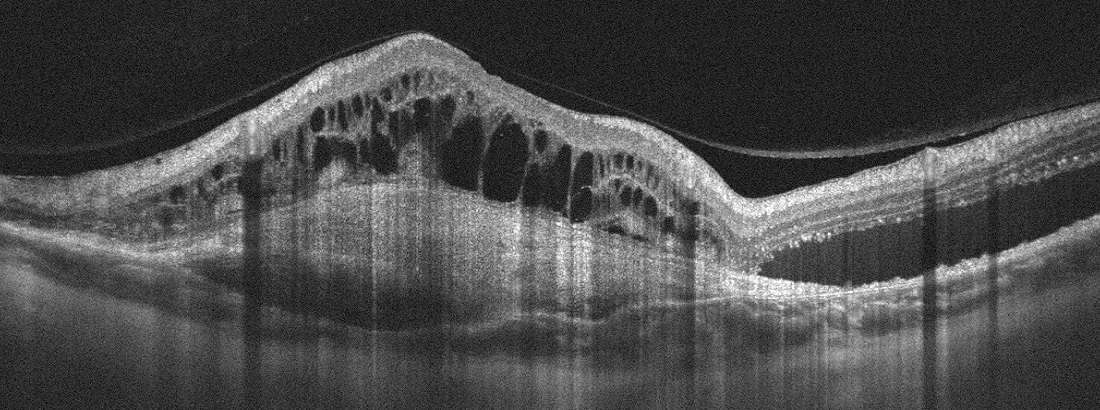 Optical coherence tomography B-scan
Finding: age-related macular degeneration (AMD).